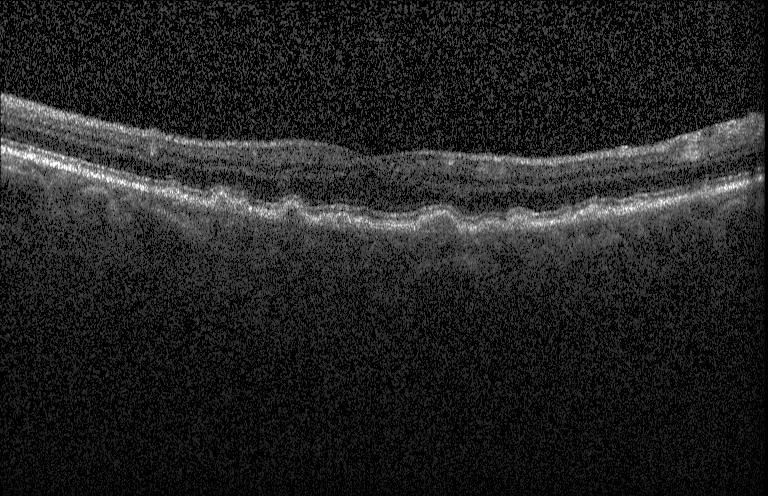 Spectral-domain OCT; optical coherence tomography scan; Heidelberg Spectralis OCT system; through the macula. Finding: multiple drusen.